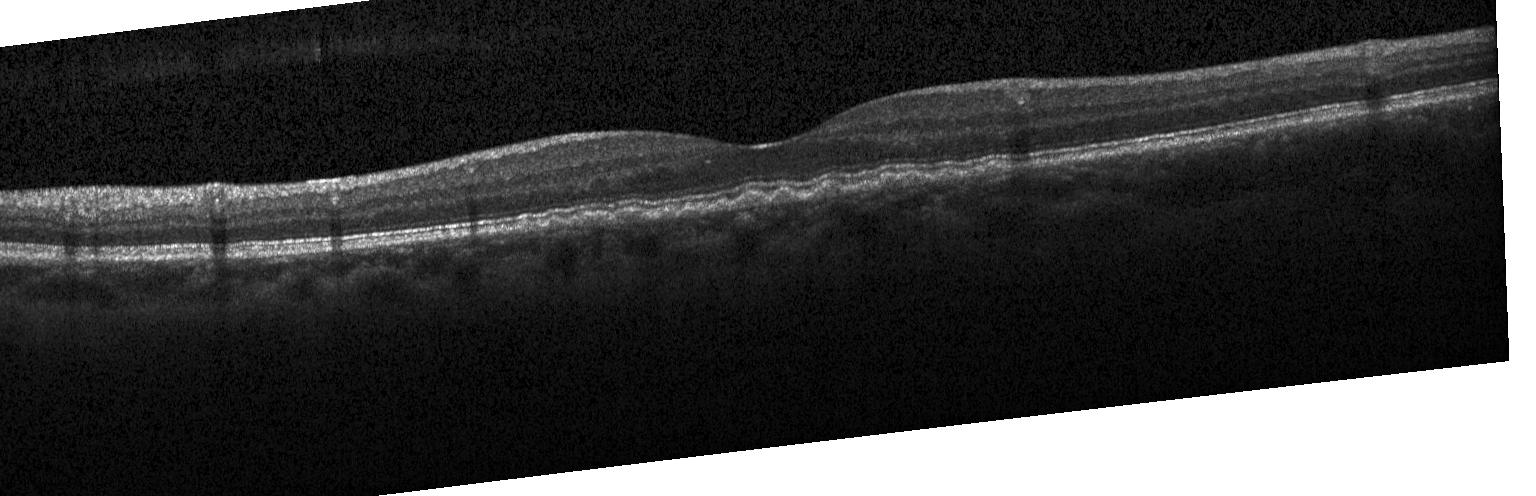 Optical coherence tomography scan; macular scan. Diagnosis: multiple drusen.